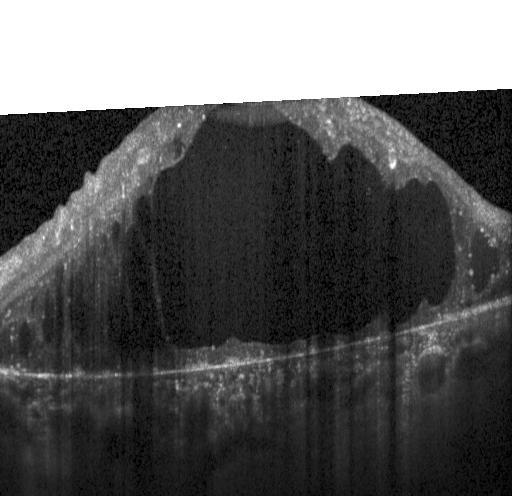 The scan shows diabetic macular edema (DME).